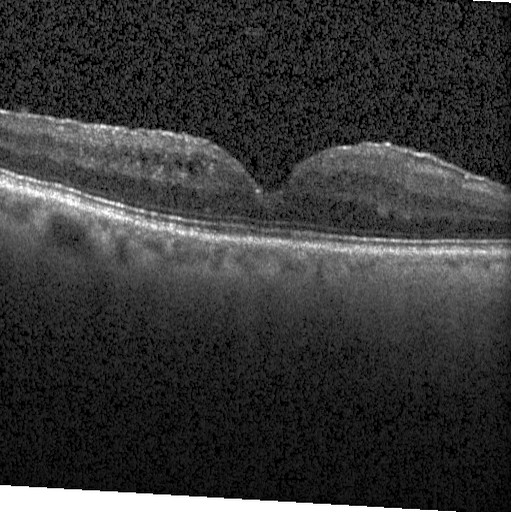
OCT B-scan. DME.